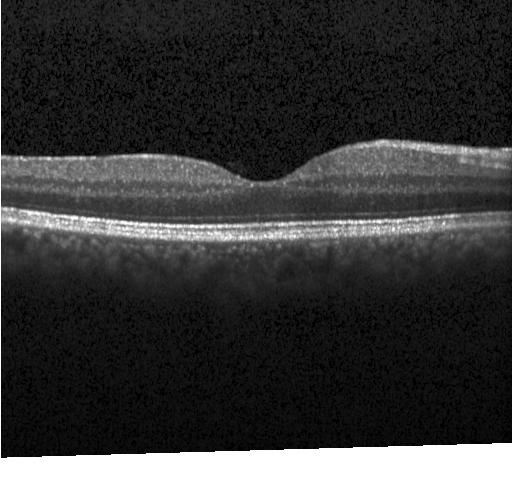
Macular OCT: no evidence of CNV, DME, or drusen.